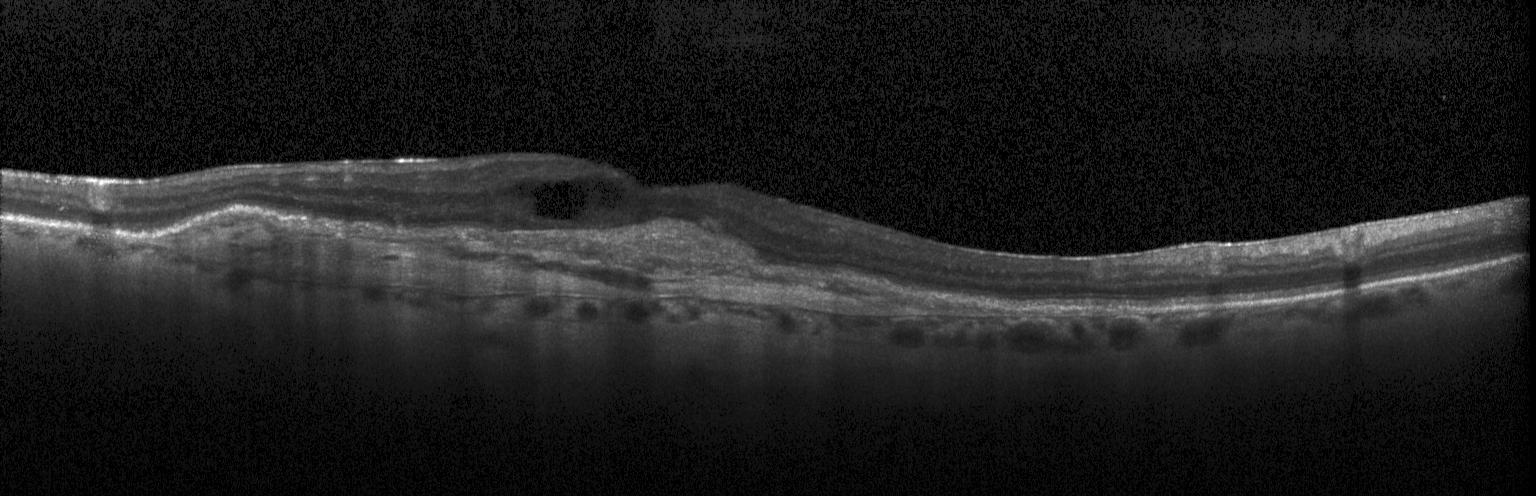 Optical coherence tomography scan.
Finding: choroidal neovascularization (CNV).